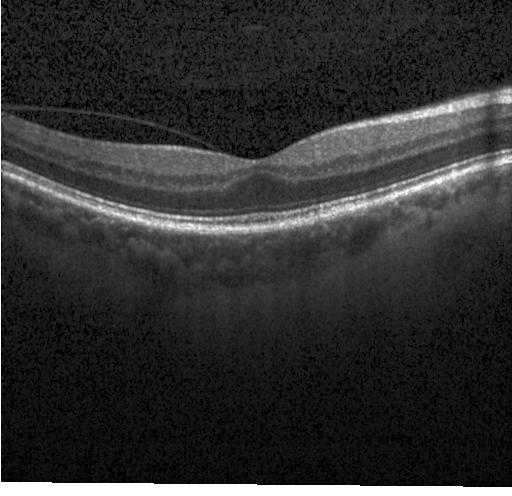
SD-OCT; fovea-centered; OCT line scan; Heidelberg Spectralis OCT system — Diagnosis: no choroidal neovascularization, no diabetic macular edema, and no drusen.